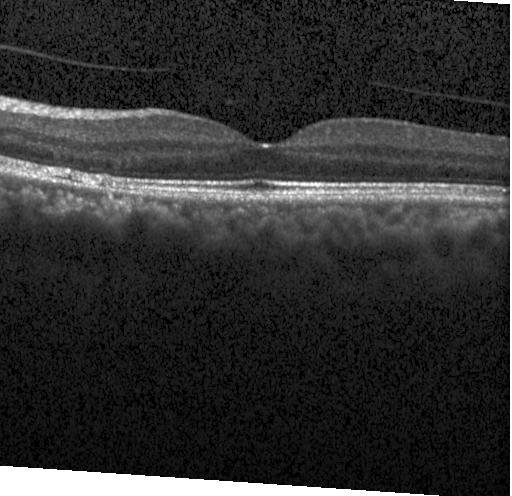
Fovea-centered · OCT line scan · SD-OCT. Impression: no choroidal neovascularization, no diabetic macular edema, and no drusen.